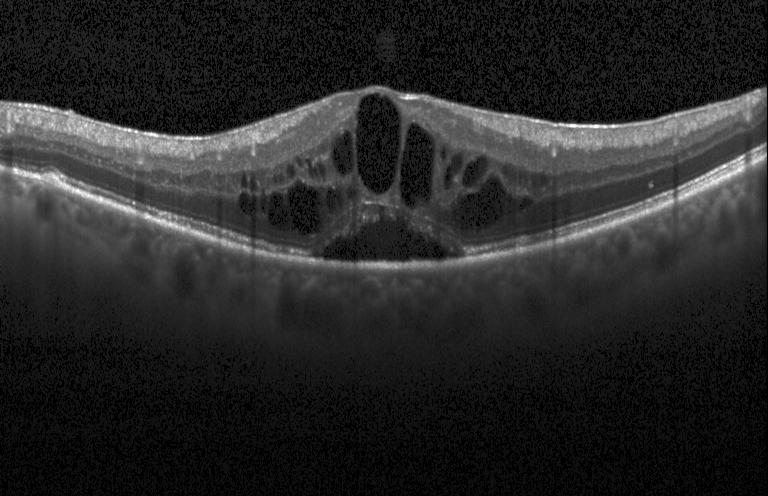
Optical coherence tomography scan. Dx: DME.